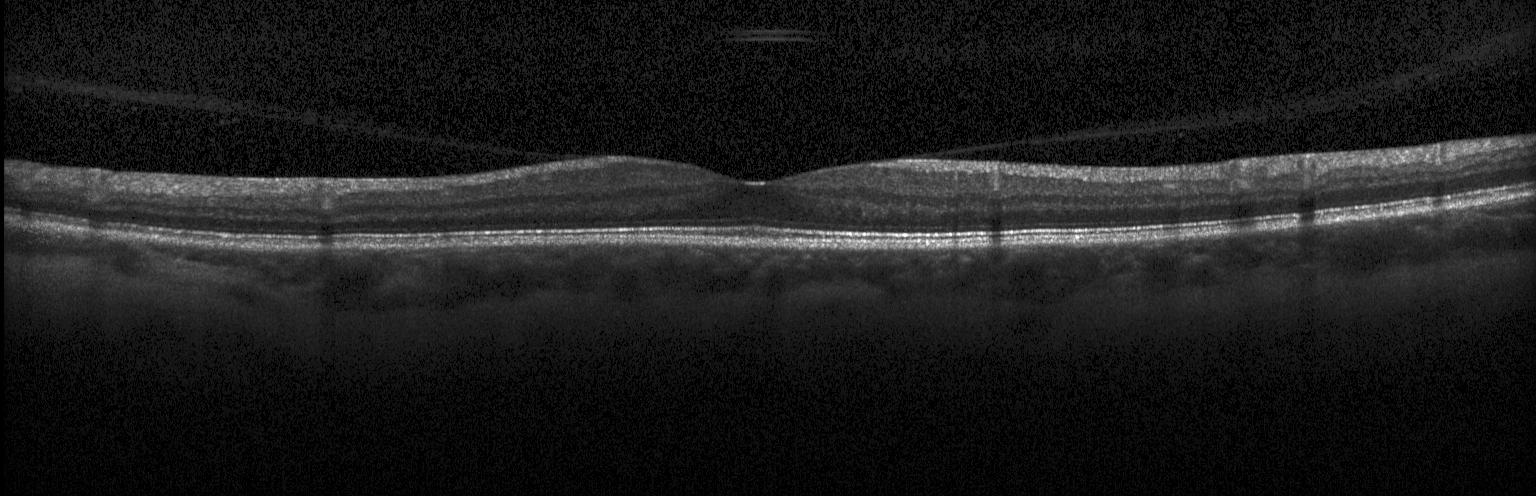 OCT B-scan. Instrument: Heidelberg Spectralis. Centered on the fovea. SD-OCT. Neither choroidal neovascularization, diabetic macular edema, nor drusen.